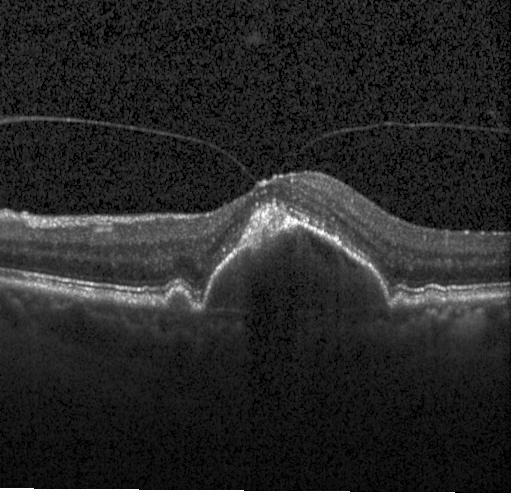
Acquired on a Heidelberg Spectralis · optical coherence tomography scan · spectral-domain OCT — Impression: choroidal neovascularization.